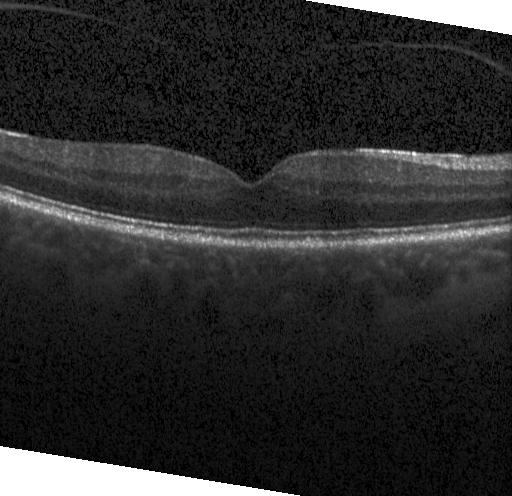

Diagnosis: neither choroidal neovascularization, diabetic macular edema, nor drusen.